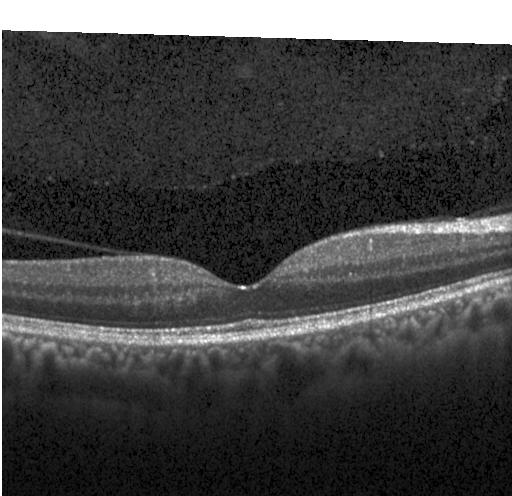
Optical coherence tomography B-scan
Impression: no CNV, DME, or drusen.